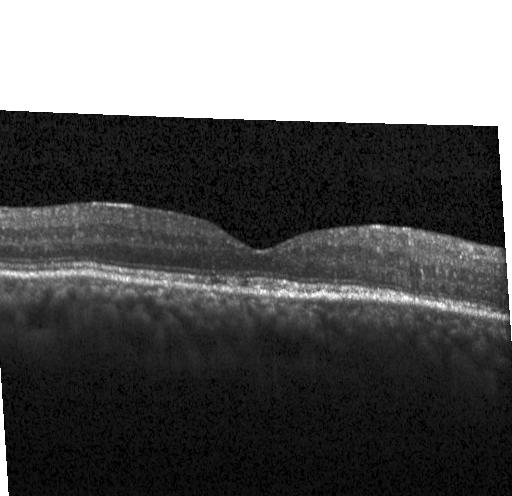 OCT finding: no choroidal neovascularization, diabetic macular edema, or drusen.